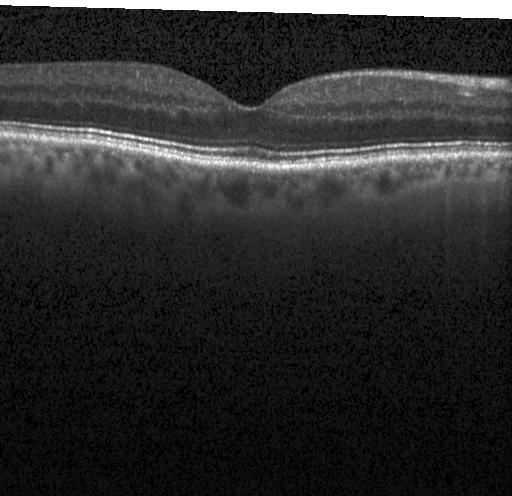 Acquired on a Heidelberg Spectralis · spectral-domain OCT · through the macula · OCT B-scan.
Impression: no CNV, DME, or drusen.